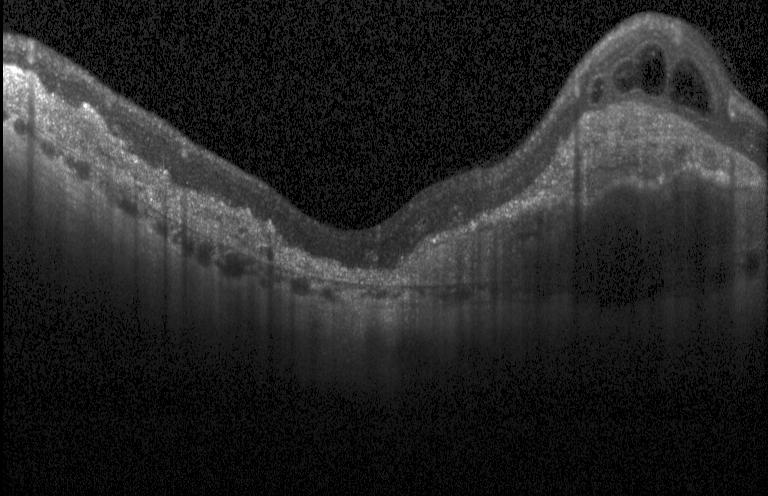 OCT scan showing a choroidal neovascular membrane.